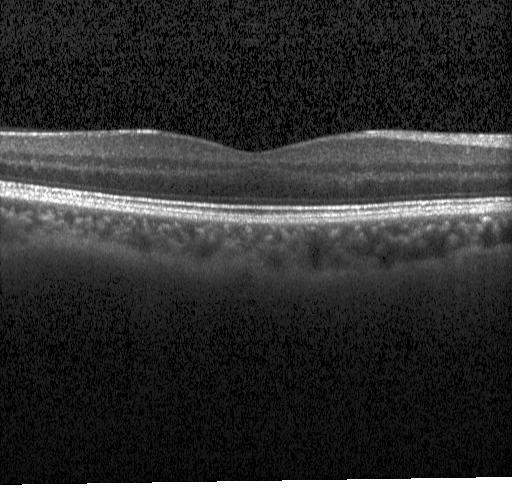
Retinal OCT cross-section showing no choroidal neovascularization, diabetic macular edema, or drusen.